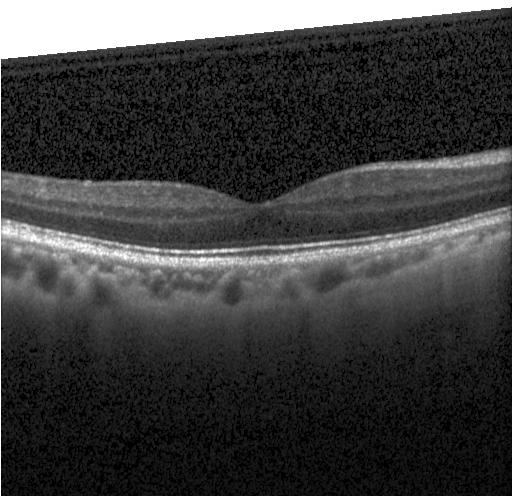
Acquired on a Heidelberg Spectralis; SD-OCT; through the macula; retinal OCT B-scan
No evidence of choroidal neovascularization, diabetic macular edema, or drusen.